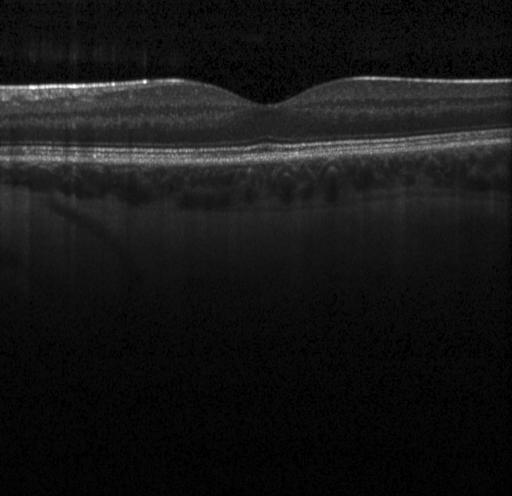
Spectral-domain OCT · retinal OCT B-scan · Heidelberg Spectralis OCT system. Diagnosis: no CNV, no DME, and no drusen.